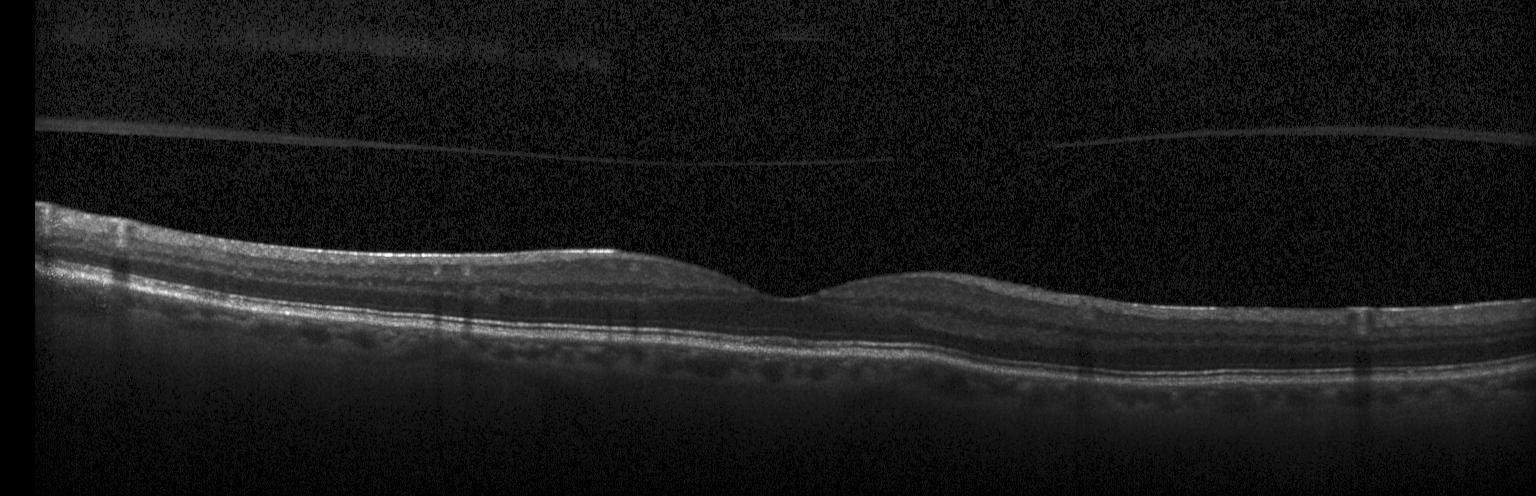

OCT B-scan, fovea-centered — Assessment: no choroidal neovascularization, no diabetic macular edema, and no drusen.